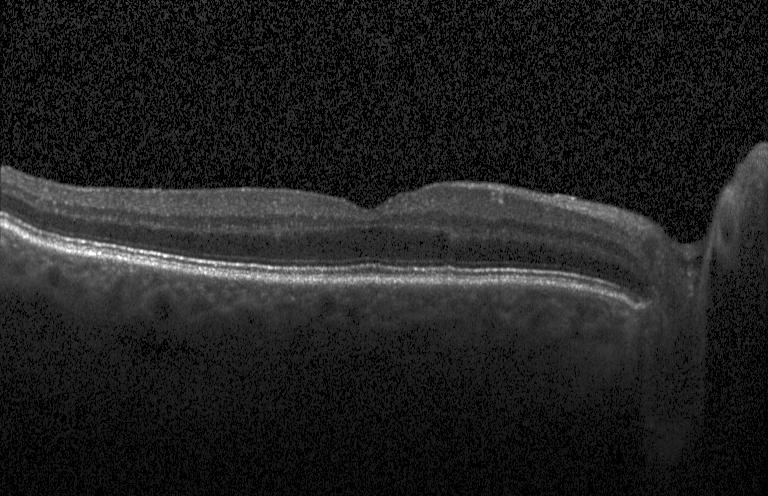

Finding: no choroidal neovascularization, diabetic macular edema, or drusen.